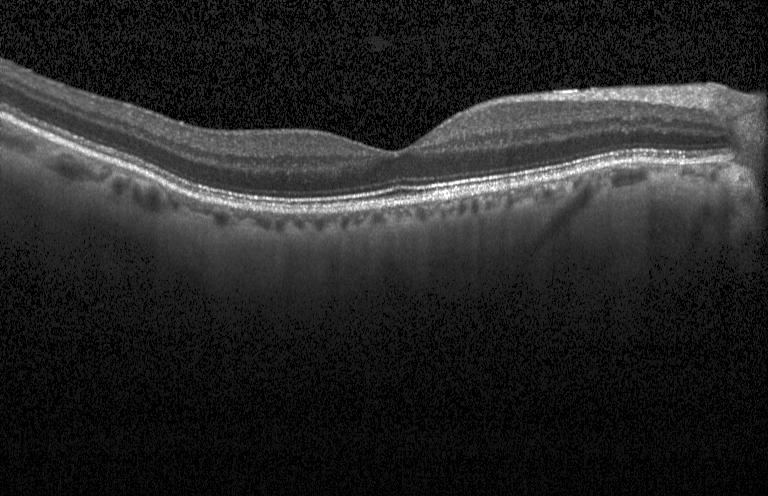 Acquired on a Heidelberg Spectralis · spectral-domain OCT · horizontal scan through the fovea · optical coherence tomography scan. Diagnosis: no choroidal neovascularization, diabetic macular edema, or drusen.